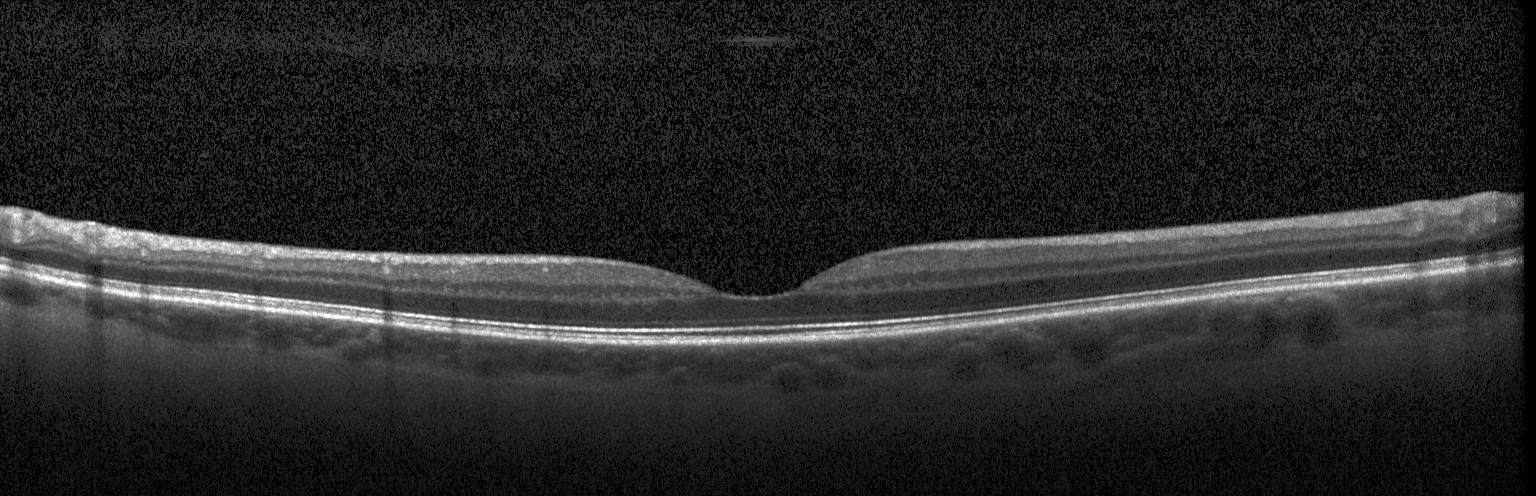

Spectral-domain optical coherence tomography, retinal OCT cross-section. Diagnosis: no evidence of choroidal neovascularization, diabetic macular edema, or drusen.